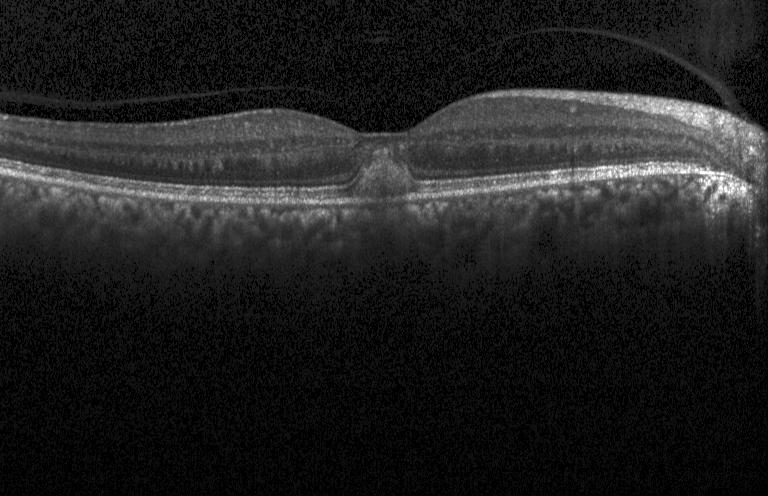
Retinal OCT B-scan; SD-OCT; macular scan; Heidelberg Spectralis. Diagnosis: a choroidal neovascular membrane.